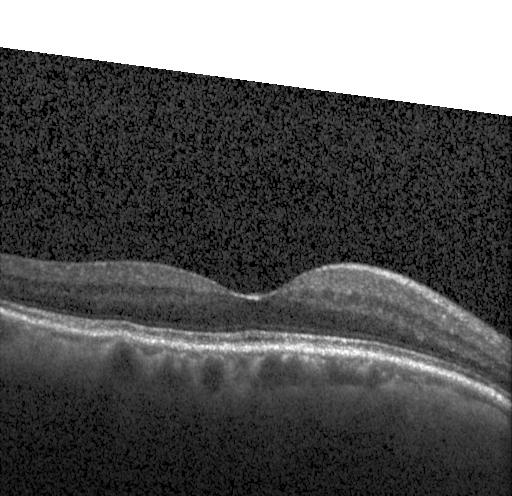 Heidelberg Spectralis OCT system; spectral-domain optical coherence tomography; optical coherence tomography scan. Diagnosis: no choroidal neovascularization, no diabetic macular edema, and no drusen.